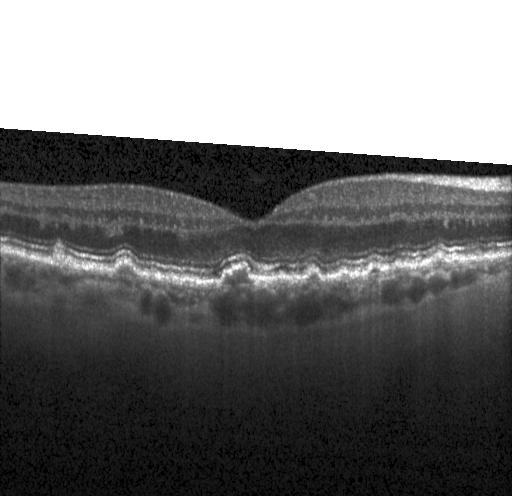

Macular OCT: multiple drusen.